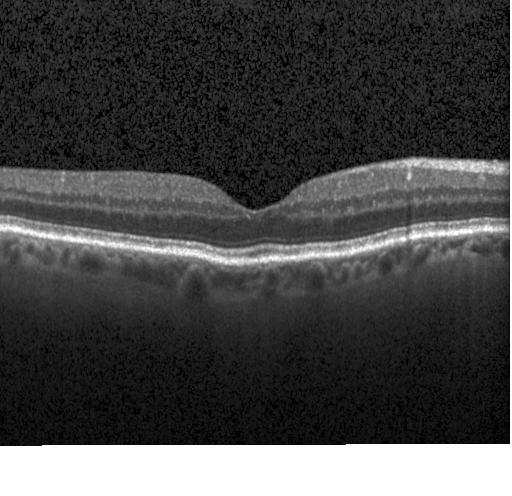 SD-OCT, centered on the fovea, Heidelberg Spectralis, OCT line scan. Assessment: no evidence of choroidal neovascularization, diabetic macular edema, or drusen.